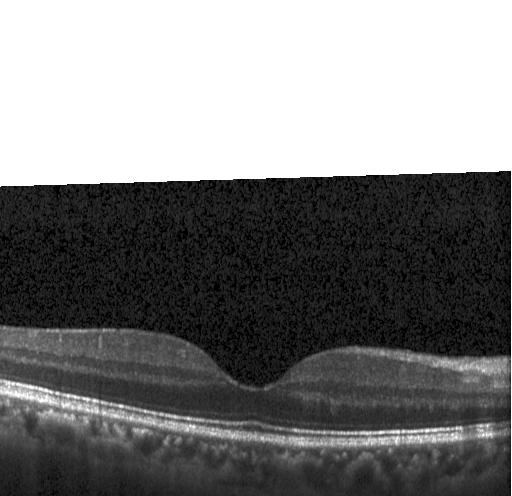 Spectral-domain optical coherence tomography · fovea-centered · instrument: Heidelberg Spectralis · optical coherence tomography B-scan.
Neither choroidal neovascularization, diabetic macular edema, nor drusen.